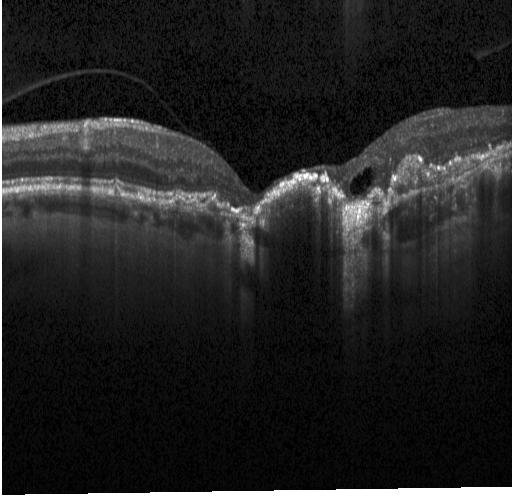

OCT scan showing CNV.